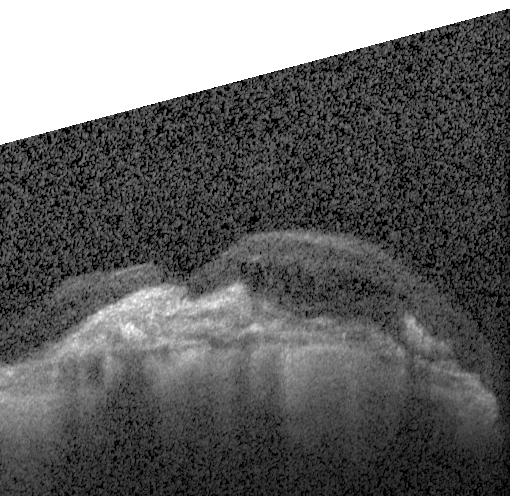 Retinal OCT B-scan; SD-OCT — Assessment: a choroidal neovascular membrane.